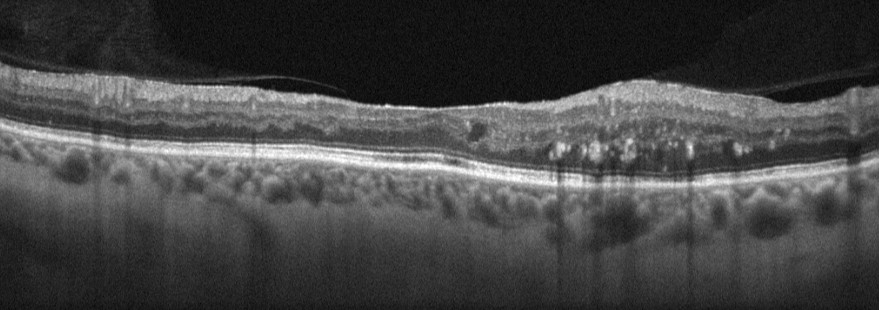

OCT B-scan. Fovea-centered — The scan shows diabetic macular edema.